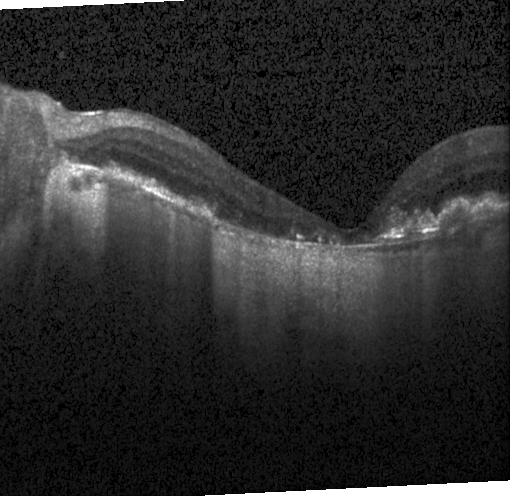
Acquired on a Heidelberg Spectralis · retinal OCT cross-section · macular scan — Impression: CNV.